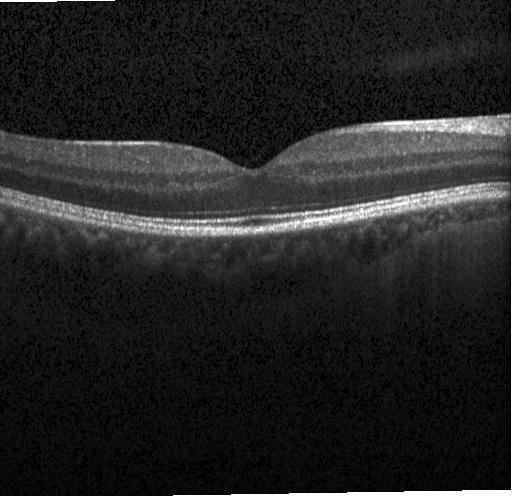
Fovea-centered. OCT line scan. Spectral-domain optical coherence tomography — No evidence of CNV, DME, or drusen.